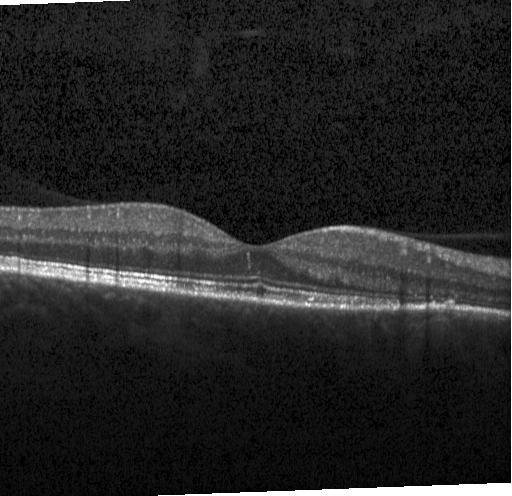
No CNV, DME, or drusen.